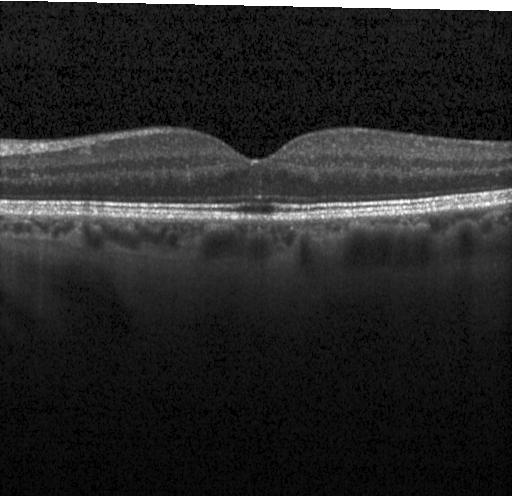 Horizontal scan through the fovea · Heidelberg Spectralis · OCT line scan · spectral-domain optical coherence tomography.
Finding: no choroidal neovascularization, no diabetic macular edema, and no drusen.